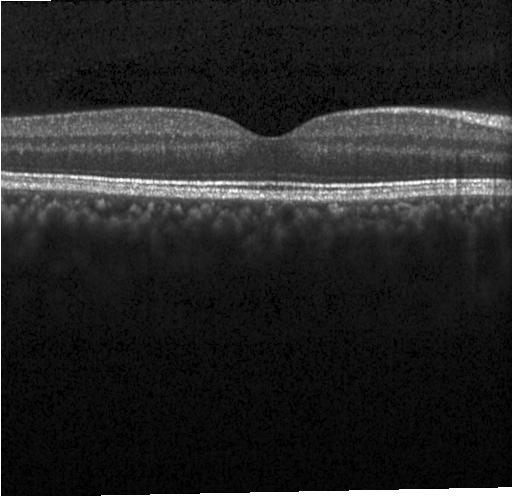 Retinal OCT cross-section showing no choroidal neovascularization, no diabetic macular edema, and no drusen.